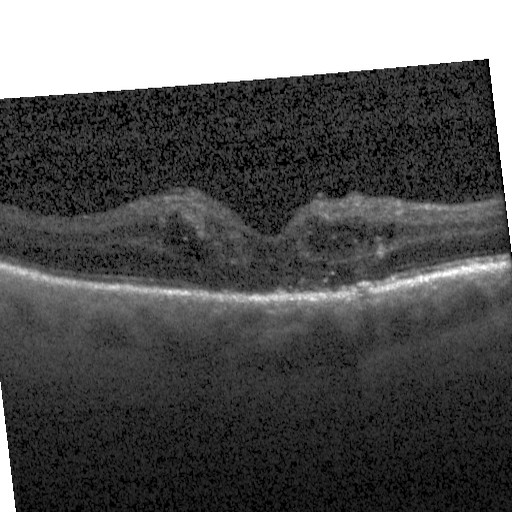
Assessment: diabetic macular edema.